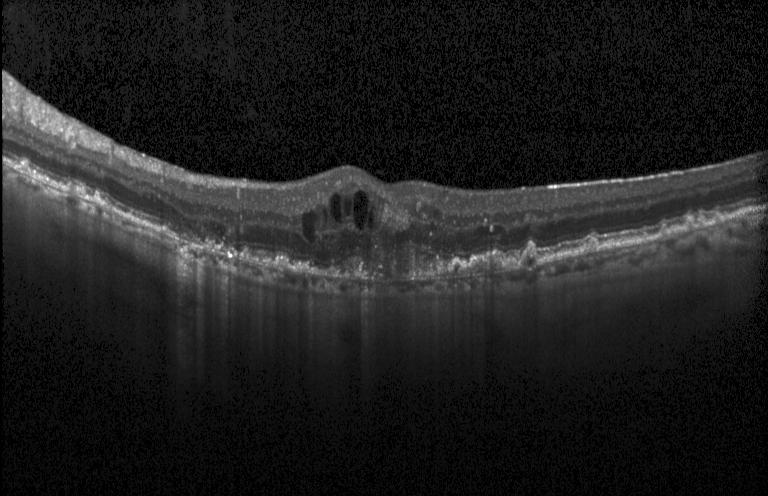

Spectral-domain optical coherence tomography. OCT line scan. Impression: a choroidal neovascular membrane.